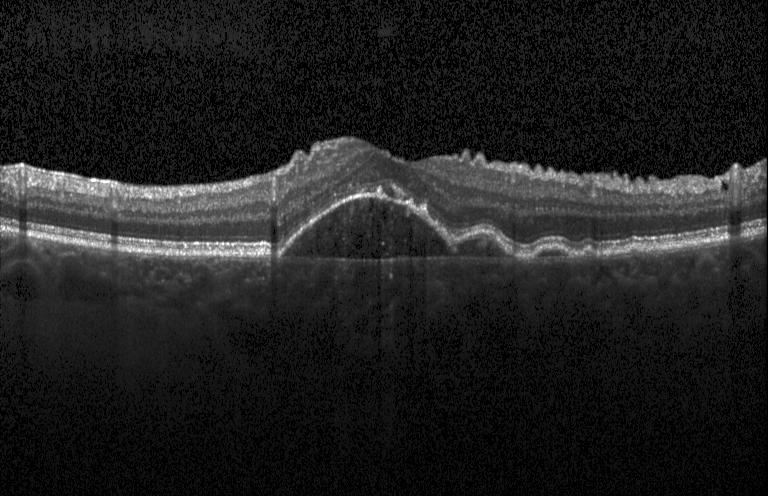 Optical coherence tomography scan. Heidelberg Spectralis. Macular scan.
OCT finding: choroidal neovascularization (CNV).